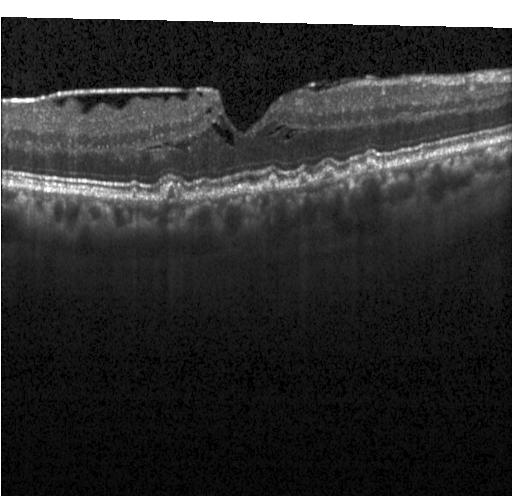 Drusen.